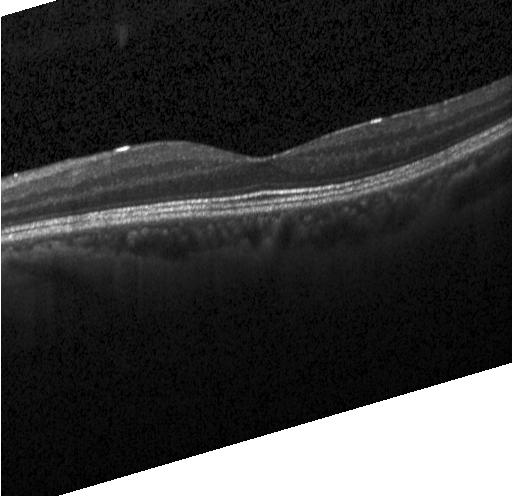
Optical coherence tomography scan — Diagnosis: neither choroidal neovascularization, diabetic macular edema, nor drusen.